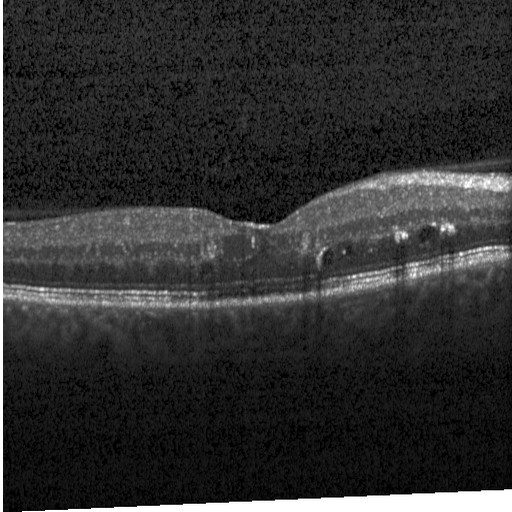

Assessment: diabetic macular edema (DME).